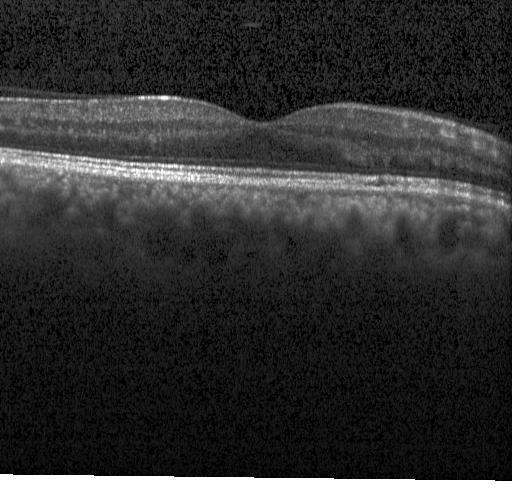

Diagnosis: no evidence of choroidal neovascularization, diabetic macular edema, or drusen.